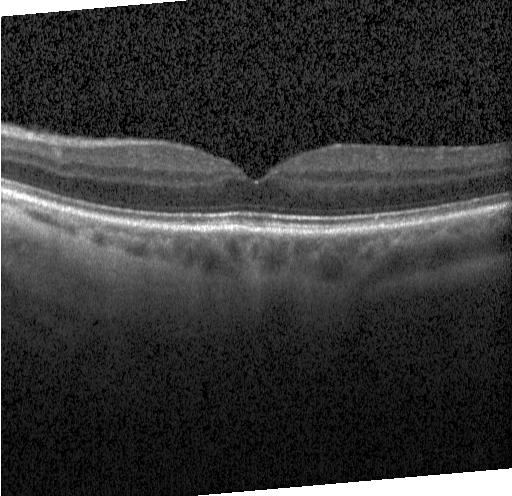

Retinal OCT cross-section — Diagnosis: neither choroidal neovascularization, diabetic macular edema, nor drusen.